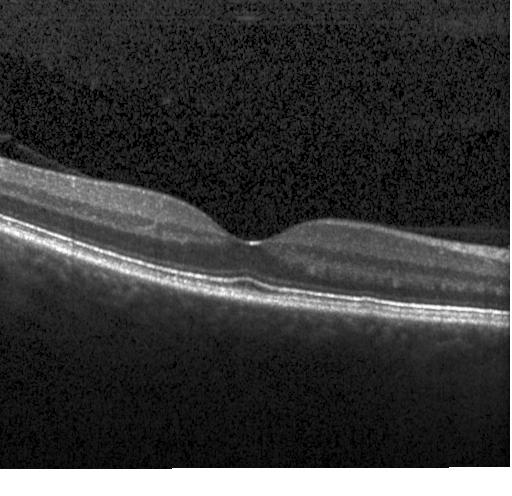
Impression: no choroidal neovascularization, no diabetic macular edema, and no drusen.